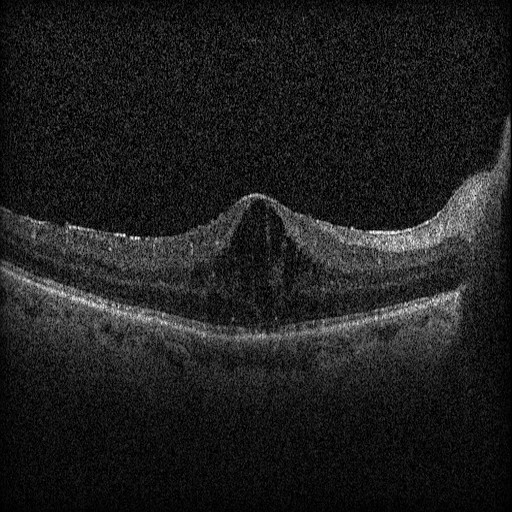

Optical coherence tomography scan · SD-OCT · instrument: Heidelberg Spectralis — The scan shows diabetic macular edema (DME).